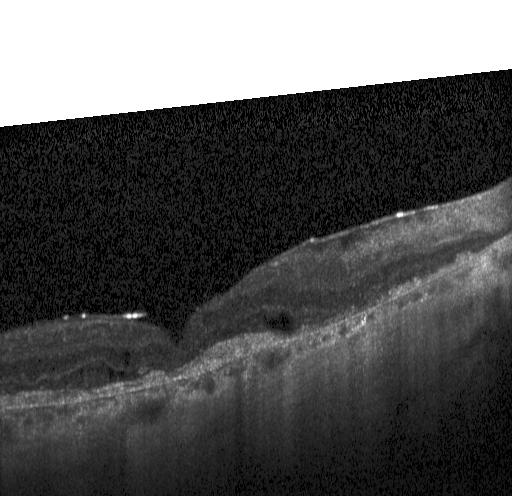
Centered on the fovea. Retinal OCT B-scan. Spectral-domain optical coherence tomography. Instrument: Heidelberg Spectralis.
Impression: a choroidal neovascular membrane.